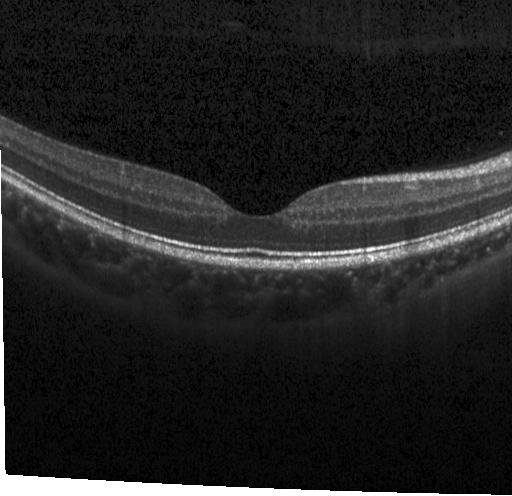 Optical coherence tomography B-scan · centered on the fovea · instrument: Heidelberg Spectralis — Assessment: no evidence of choroidal neovascularization, diabetic macular edema, or drusen.